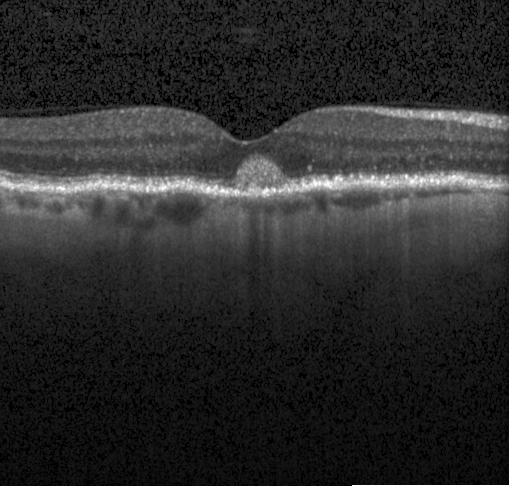 Spectral-domain optical coherence tomography, optical coherence tomography scan. Diagnosis: multiple drusen.